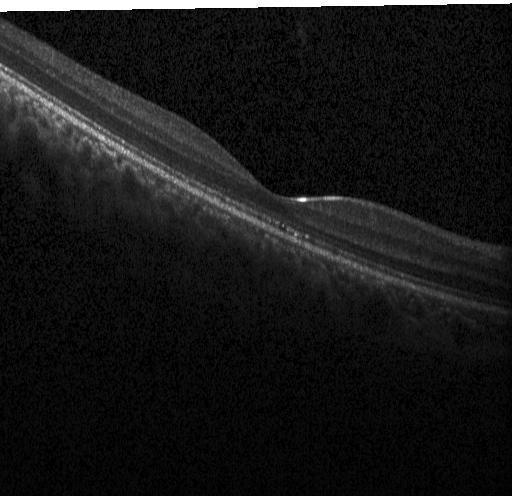 Optical coherence tomography B-scan — Diagnosis: no evidence of choroidal neovascularization, diabetic macular edema, or drusen.